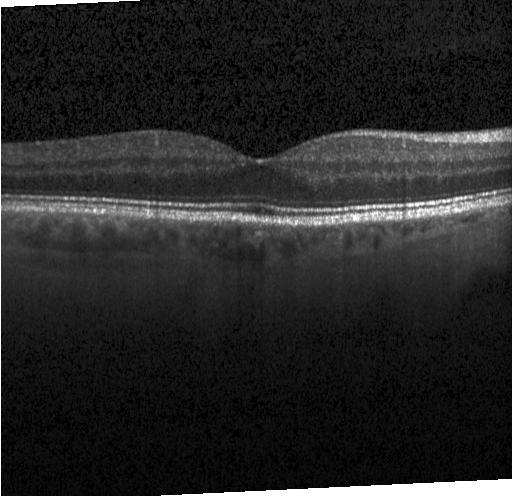

Macular OCT demonstrating neither CNV, DME, nor drusen.